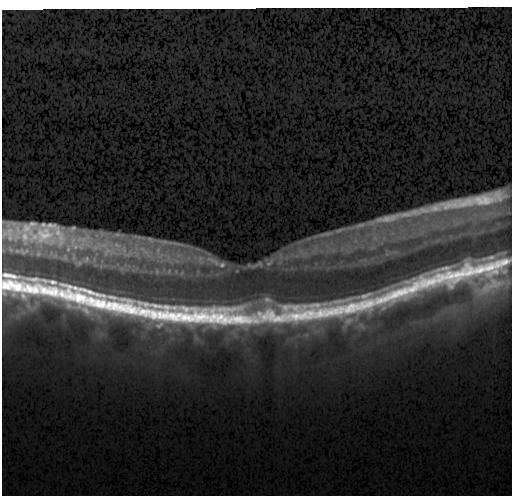 Finding: drusen.